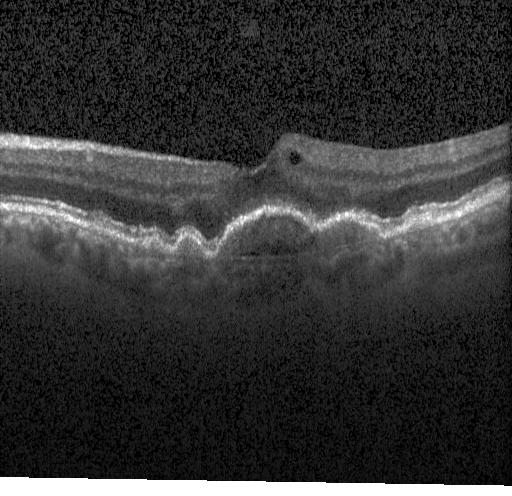

Impression: a choroidal neovascular membrane.